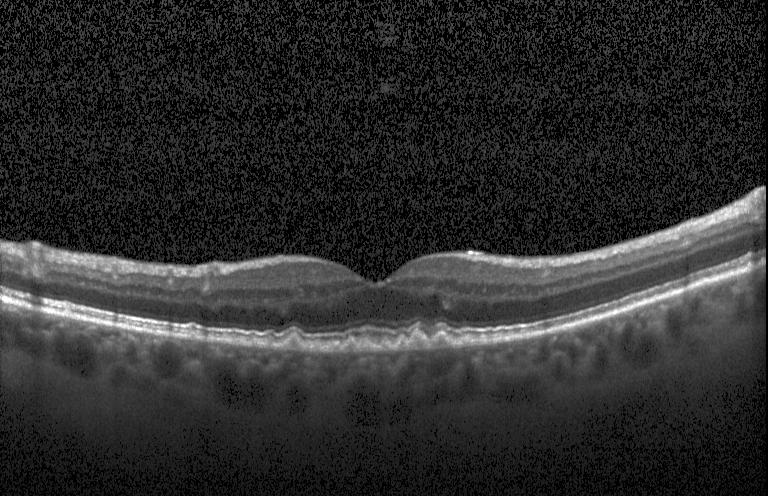 OCT line scan. Heidelberg Spectralis. Horizontal scan through the fovea
Impression: drusen.